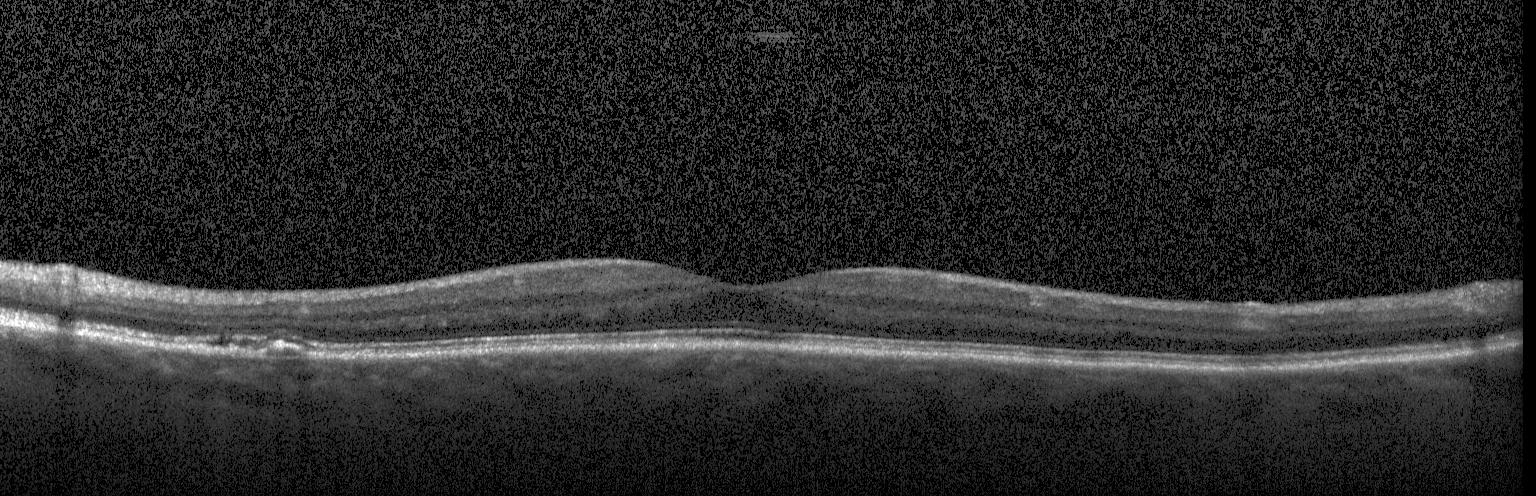

Retinal OCT B-scan
Diagnosis: choroidal neovascularization.